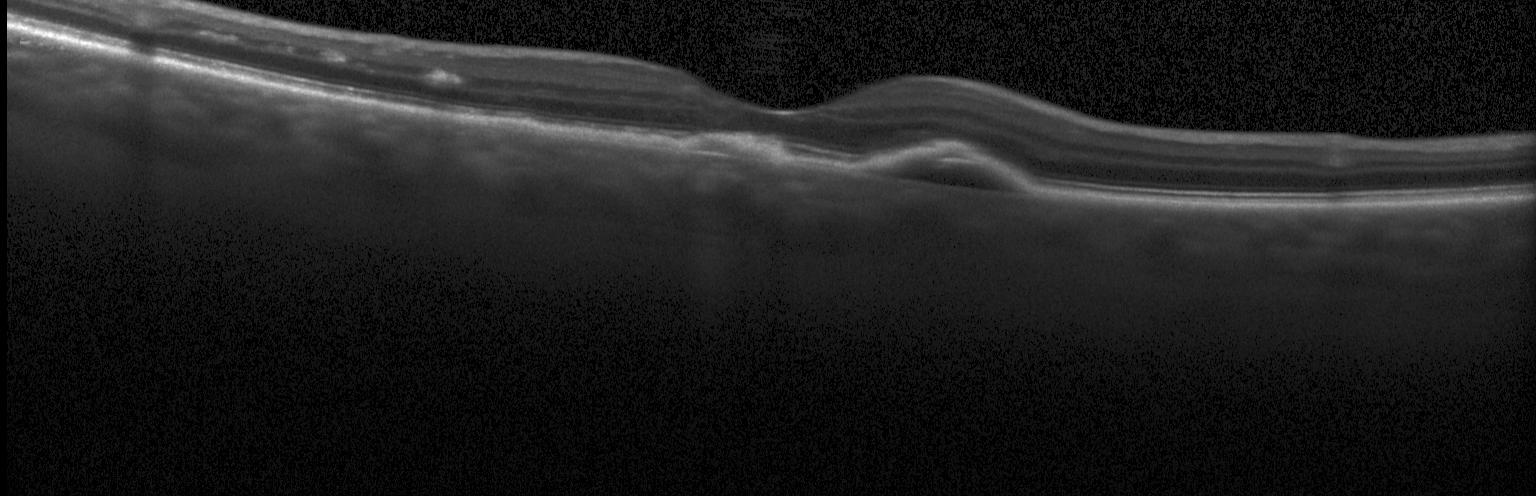
OCT line scan. Heidelberg Spectralis. SD-OCT — Assessment: choroidal neovascularization (CNV).